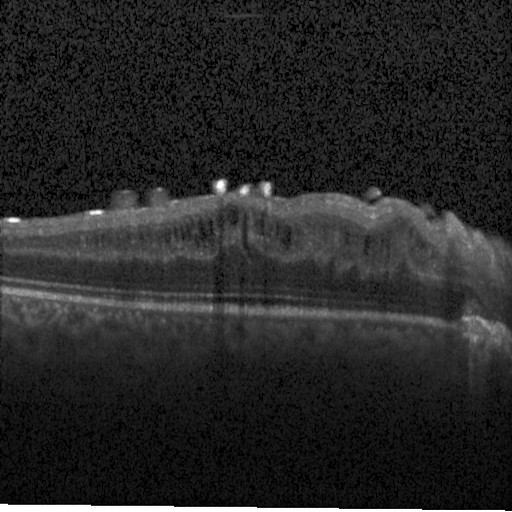

OCT line scan. The scan shows DME.